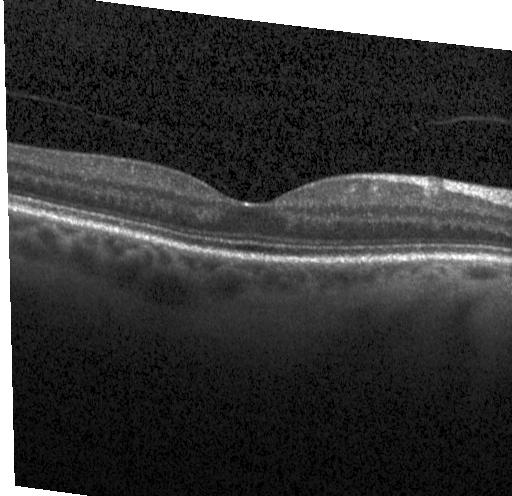

Finding: no choroidal neovascularization, no diabetic macular edema, and no drusen.